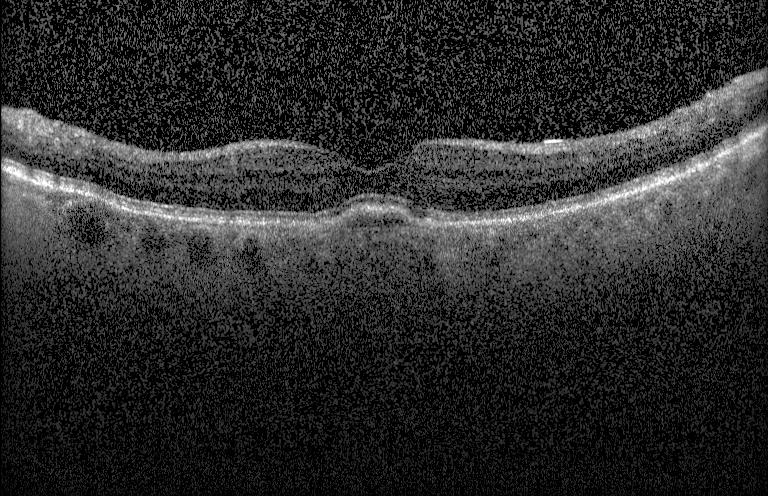

Finding: a choroidal neovascular membrane.